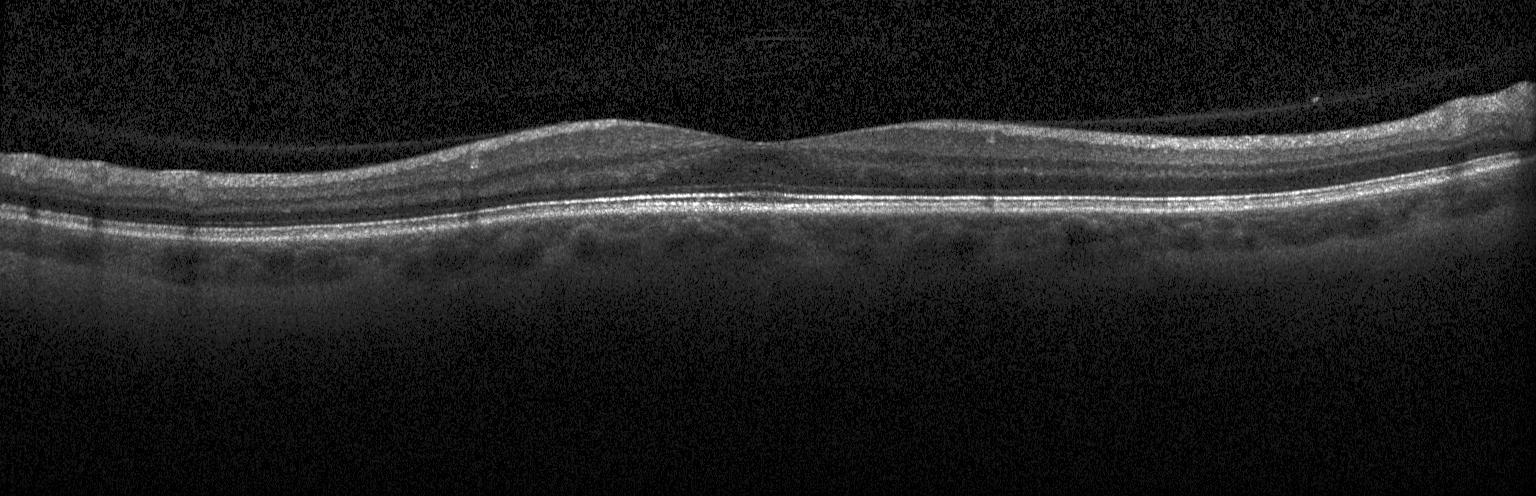
Heidelberg Spectralis OCT system. SD-OCT. OCT line scan.
Impression: neither choroidal neovascularization, diabetic macular edema, nor drusen.